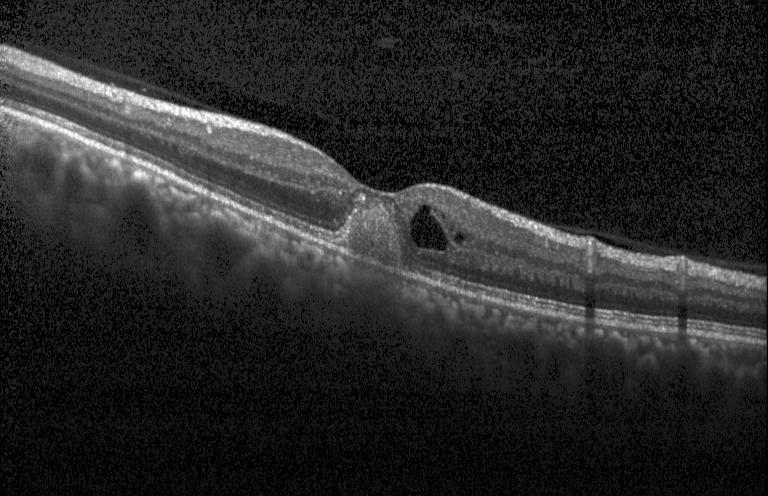
OCT scan showing a choroidal neovascular membrane.